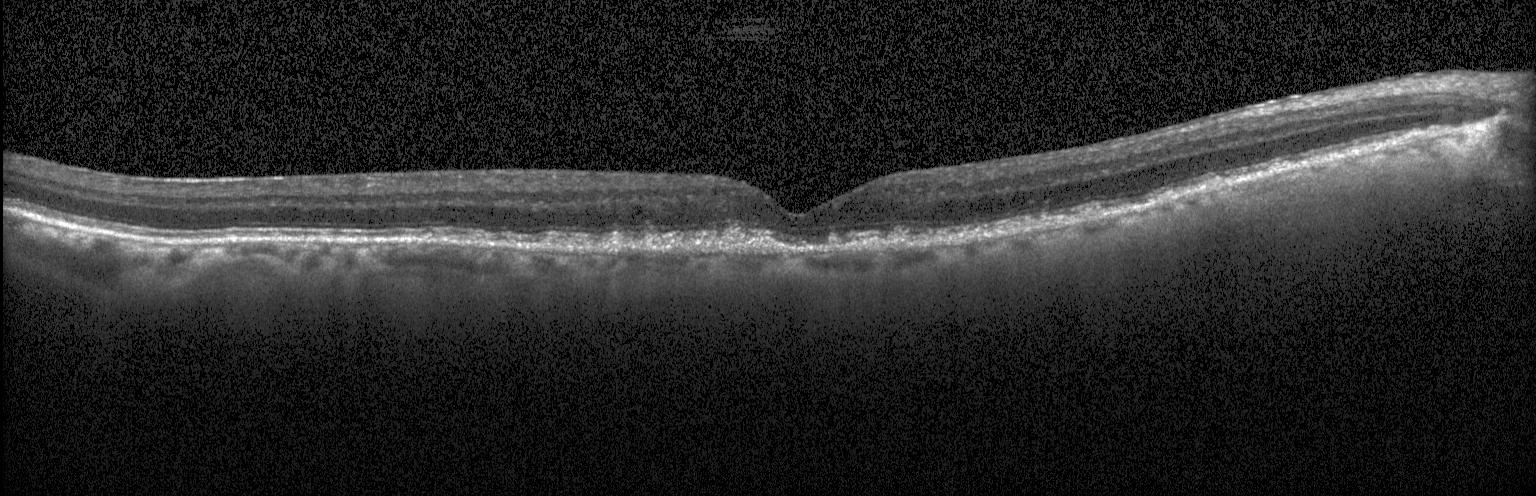

Assessment: sub-RPE drusenoid deposits.